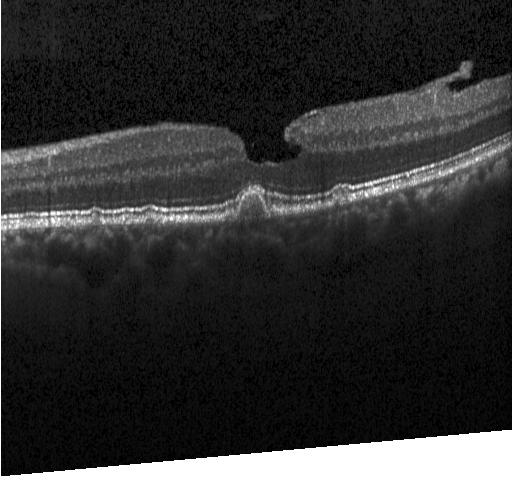 Fovea-centered · OCT line scan.
Impression: multiple drusen.